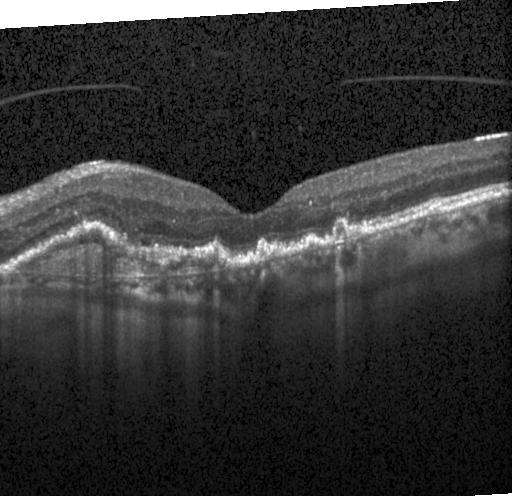
OCT B-scan. Spectral-domain OCT. Through the macula — CNV.